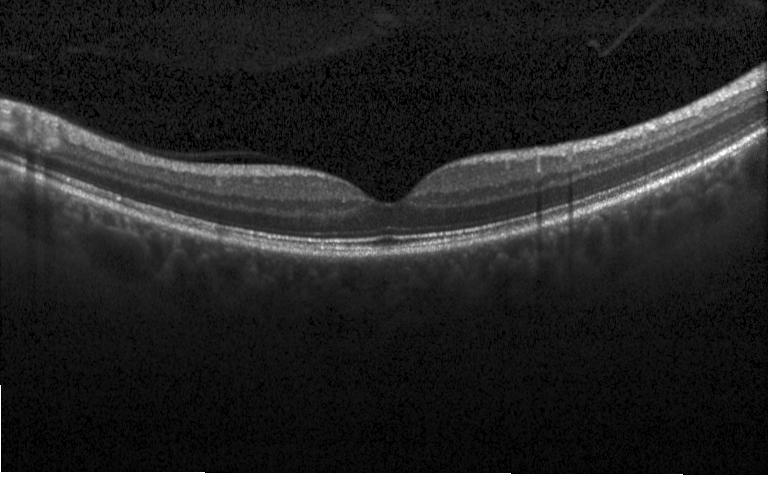 OCT B-scan showing no choroidal neovascularization, no diabetic macular edema, and no drusen.